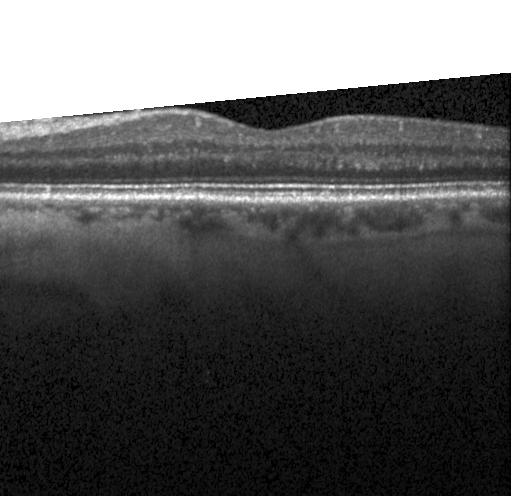

OCT line scan; macular scan; spectral-domain OCT; instrument: Heidelberg Spectralis
Diagnosis: no choroidal neovascularization, no diabetic macular edema, and no drusen.